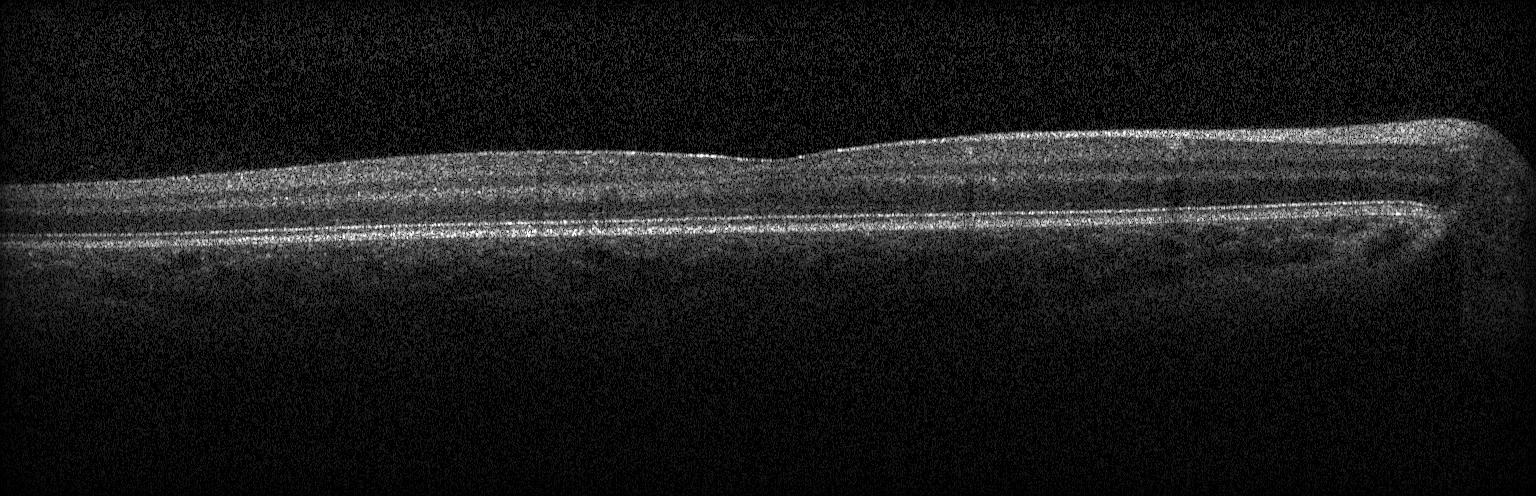

No evidence of CNV, DME, or drusen.